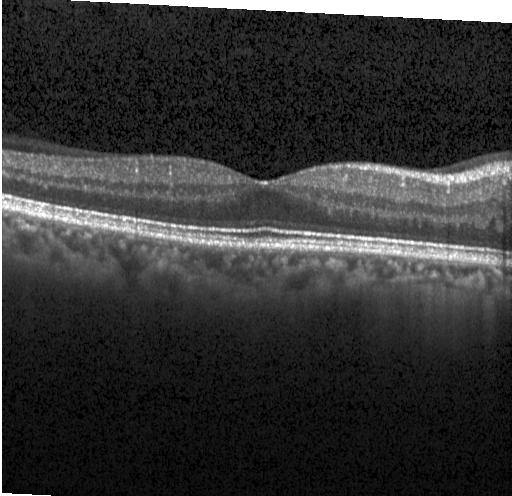 Finding: neither choroidal neovascularization, diabetic macular edema, nor drusen.